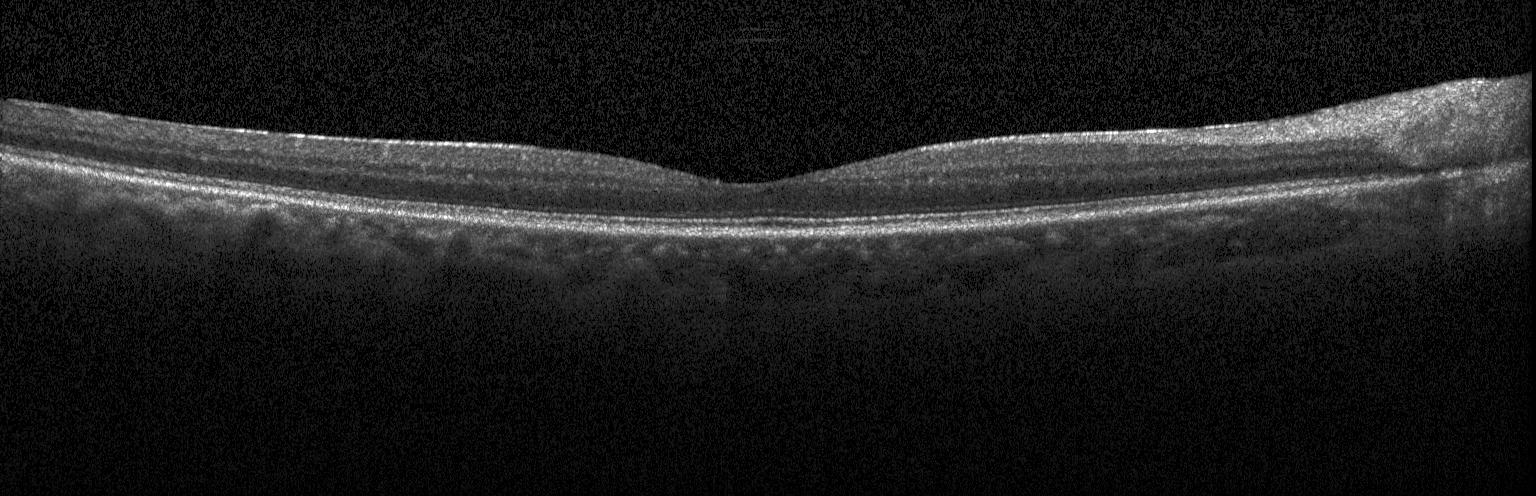 Assessment: no CNV, DME, or drusen.